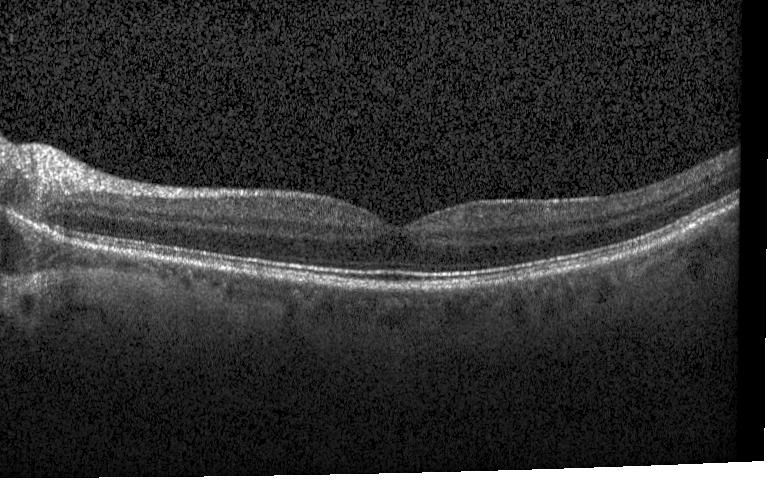

Diagnosis: no choroidal neovascularization, diabetic macular edema, or drusen.